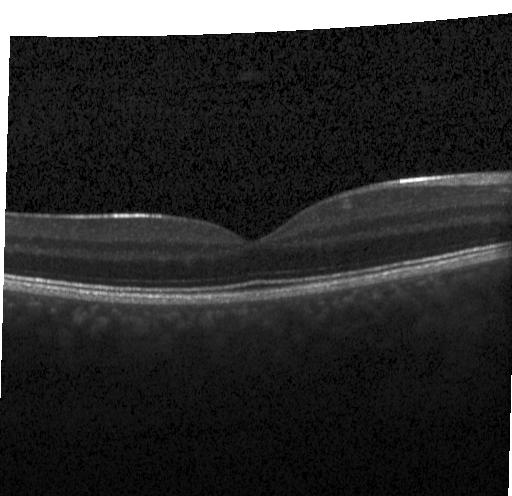 Macular OCT demonstrating neither choroidal neovascularization, diabetic macular edema, nor drusen.